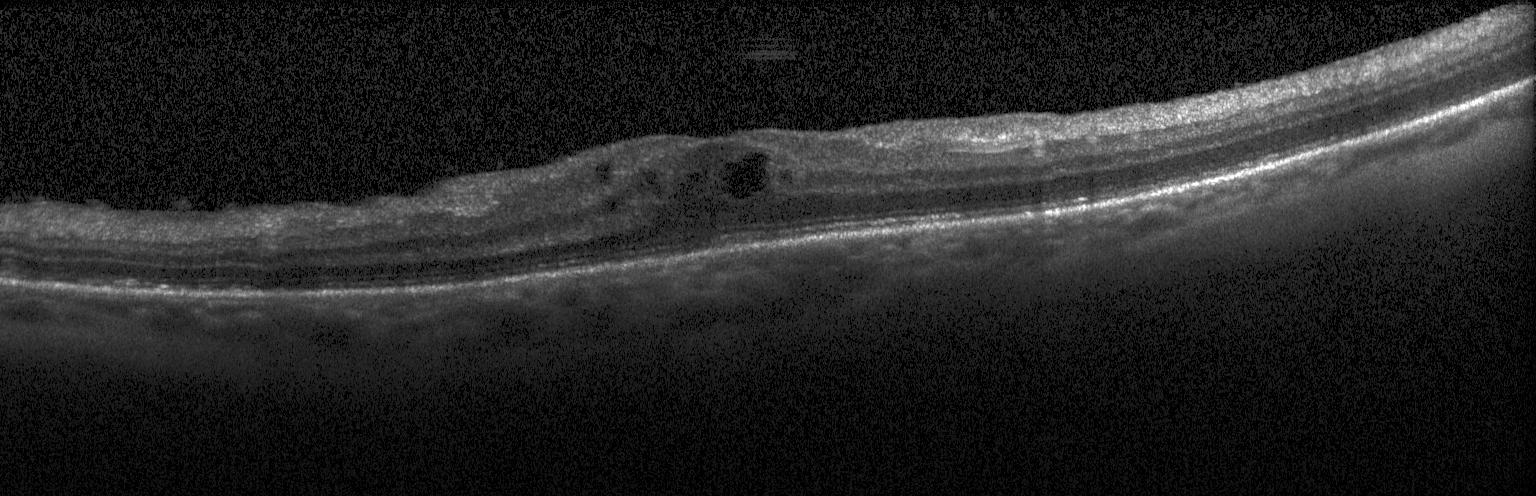
Impression: DME.